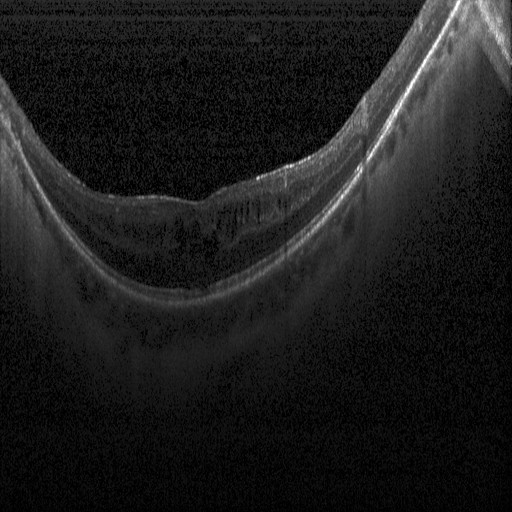
OCT B-scan showing DME.